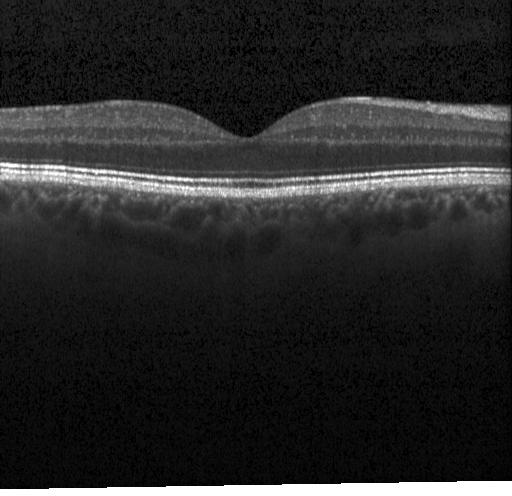 Dx: no CNV, no DME, and no drusen.